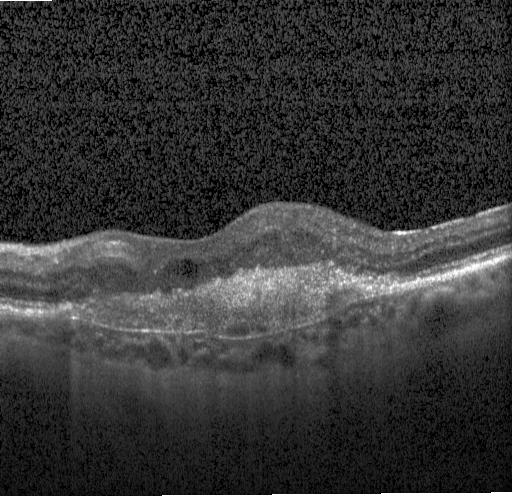
This B-scan demonstrates a choroidal neovascular membrane.